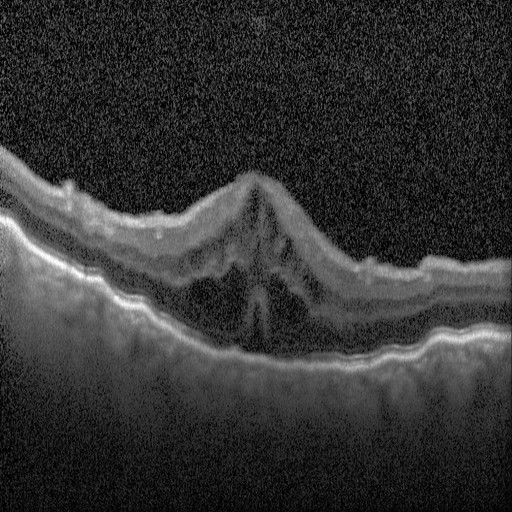

Acquired on a Heidelberg Spectralis. Retinal OCT B-scan
Diagnosis: diabetic macular edema (DME).